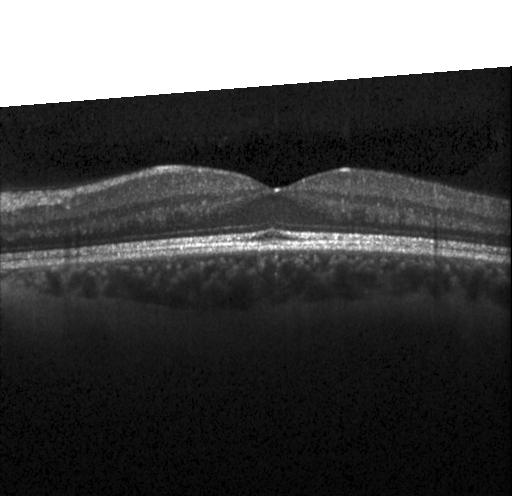
Retinal OCT cross-section. Instrument: Heidelberg Spectralis.
Diagnosis: neither choroidal neovascularization, diabetic macular edema, nor drusen.